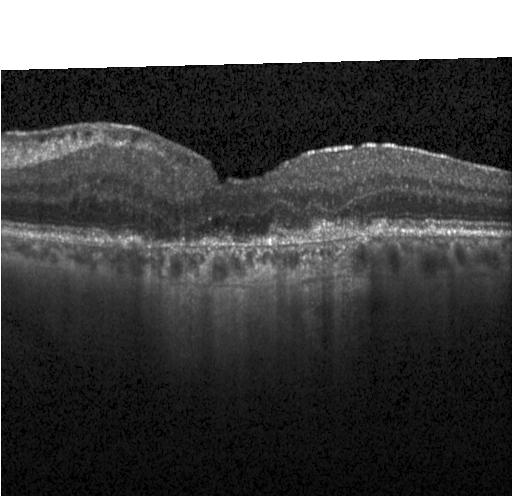 Spectral-domain OCT. Retinal OCT cross-section — Assessment: choroidal neovascularization.